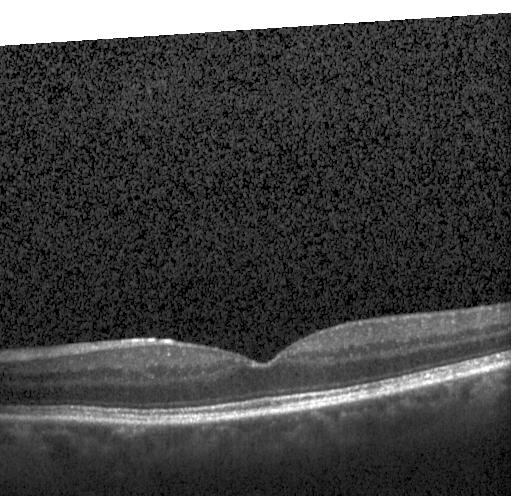
OCT B-scan
Finding: neither choroidal neovascularization, diabetic macular edema, nor drusen.